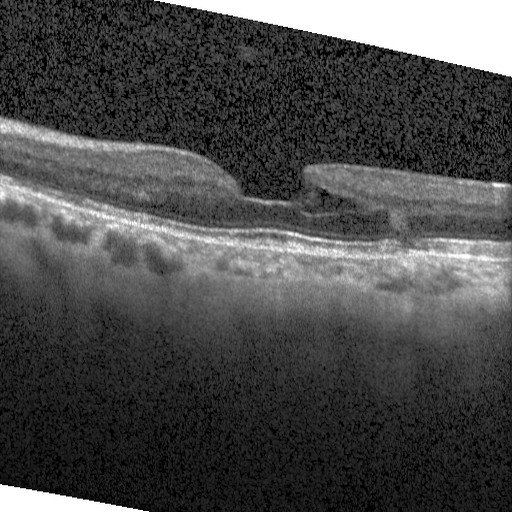

Instrument: Heidelberg Spectralis, OCT B-scan, spectral-domain OCT, horizontal scan through the fovea.
OCT finding: DME.